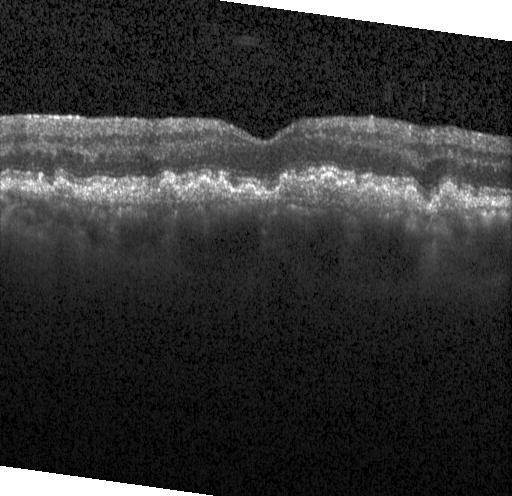 Optical coherence tomography scan — Finding: a choroidal neovascular membrane.